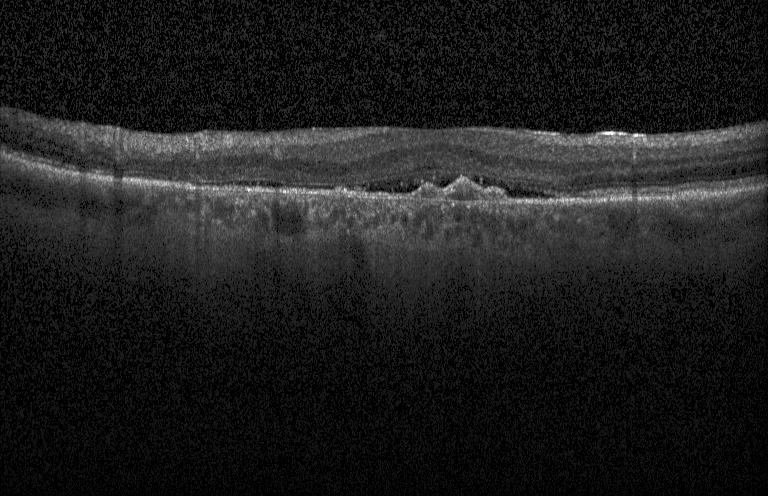
Retinal OCT cross-section showing choroidal neovascularization (CNV).